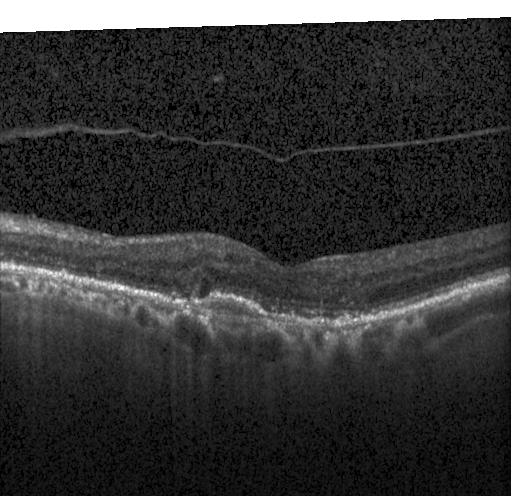
Assessment: a choroidal neovascular membrane.